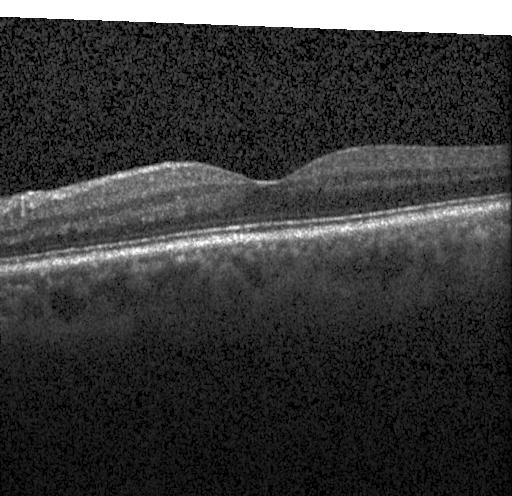

Instrument: Heidelberg Spectralis · macular scan · spectral-domain optical coherence tomography · retinal OCT B-scan. Impression: no evidence of CNV, DME, or drusen.